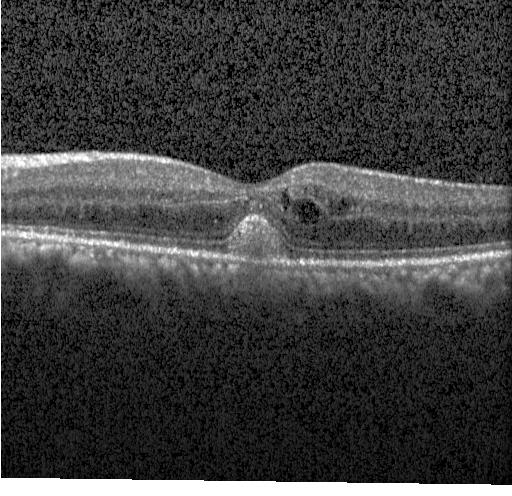 Acquired on a Heidelberg Spectralis · SD-OCT · retinal OCT cross-section — This B-scan demonstrates a choroidal neovascular membrane.